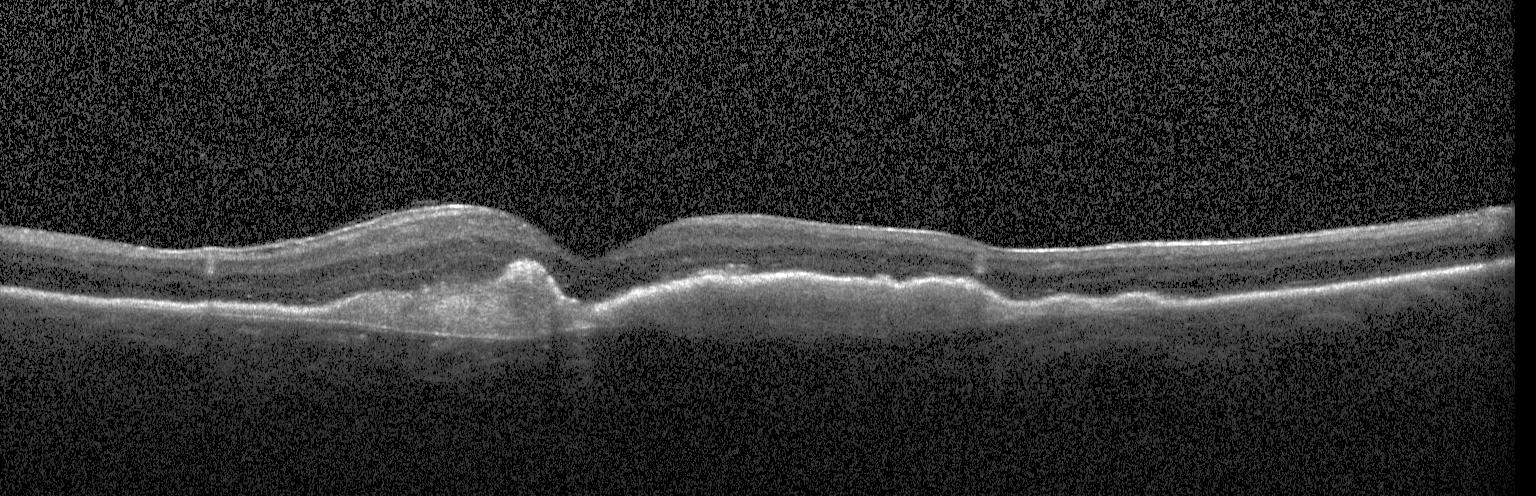

Horizontal scan through the fovea · Heidelberg Spectralis · SD-OCT · optical coherence tomography scan.
Diagnosis: a choroidal neovascular membrane.